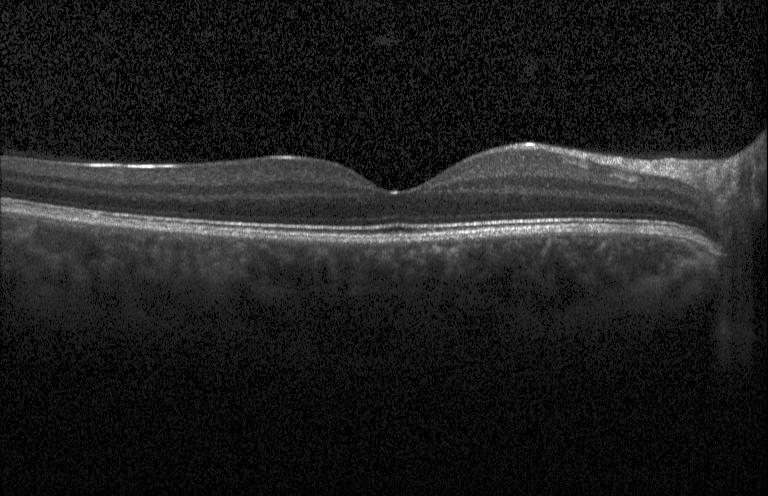
Spectral-domain OCT B-scan: neither choroidal neovascularization, diabetic macular edema, nor drusen.